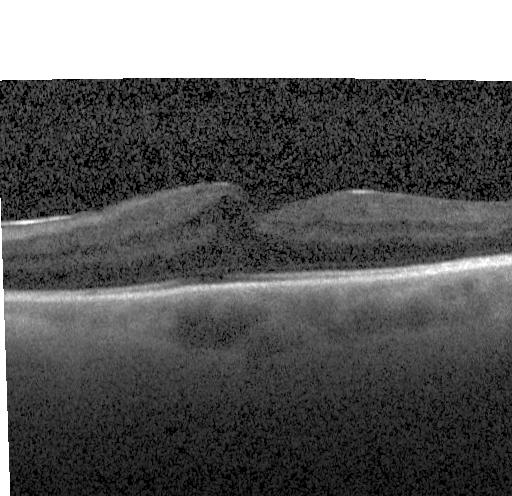

Diagnosis: diabetic macular edema.